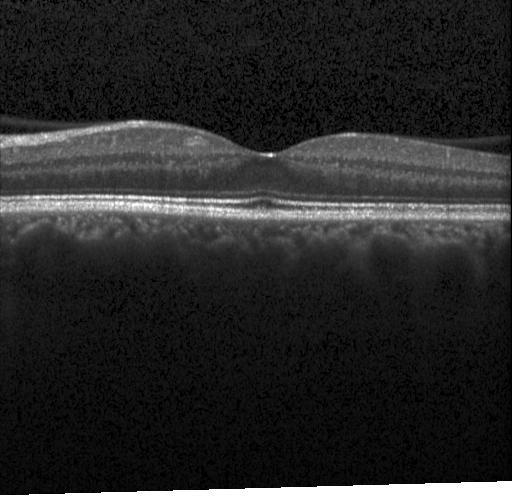
Macular OCT: no evidence of choroidal neovascularization, diabetic macular edema, or drusen.